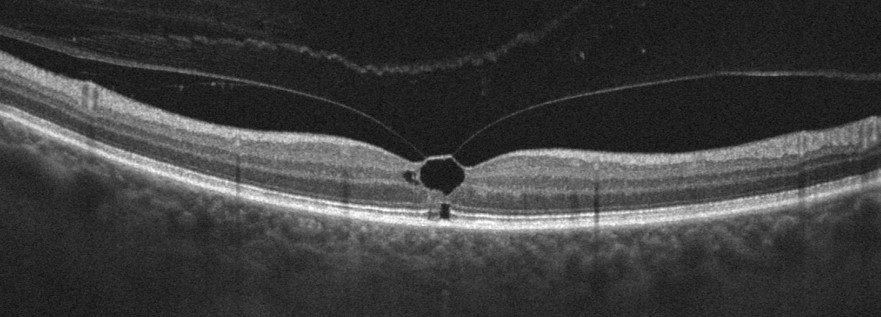

Dx: vitreomacular interface disease.